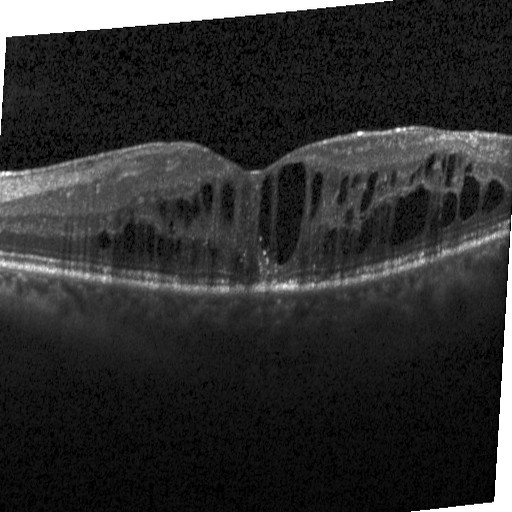 Instrument: Heidelberg Spectralis; optical coherence tomography B-scan — Dx: diabetic macular edema.